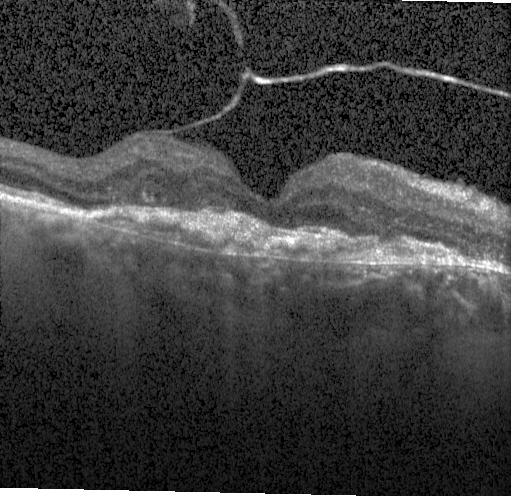 Horizontal scan through the fovea · OCT line scan. The scan shows choroidal neovascularization.